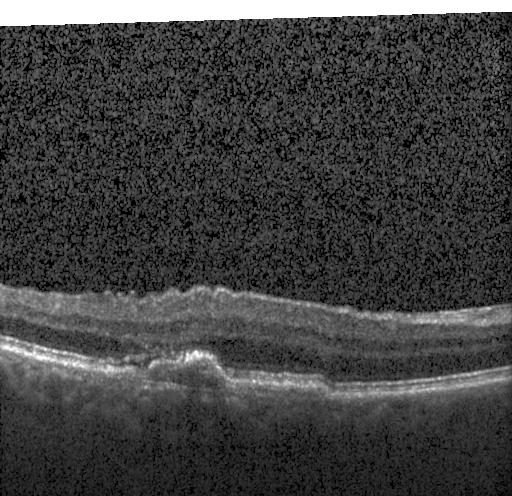 OCT finding: CNV.